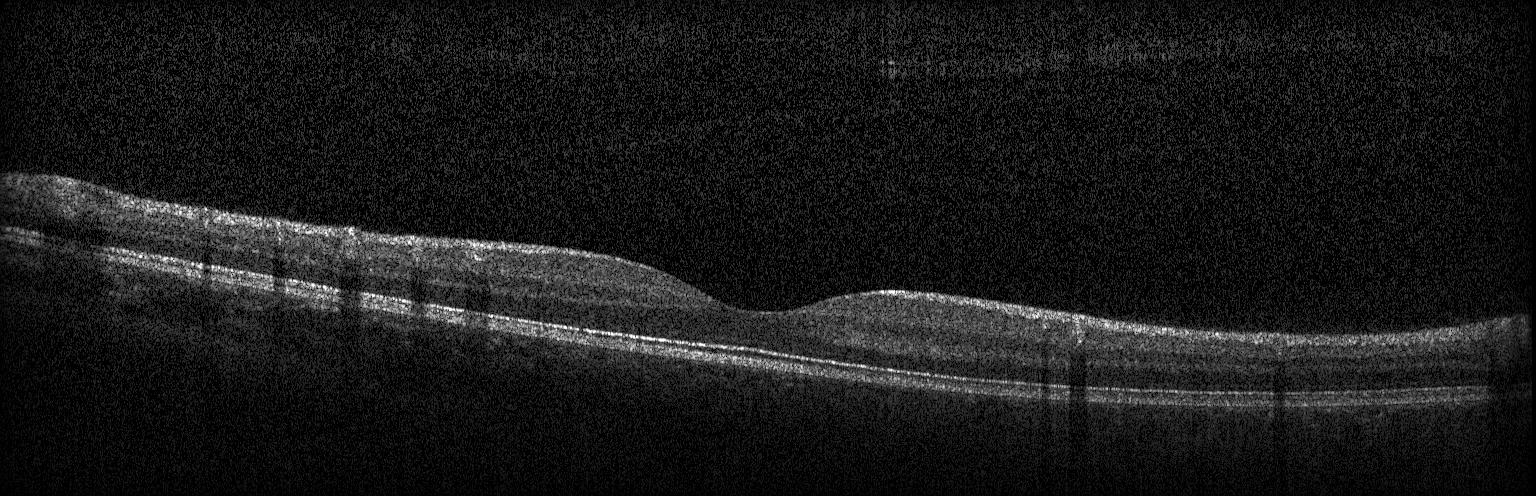 OCT scan showing no choroidal neovascularization, no diabetic macular edema, and no drusen.